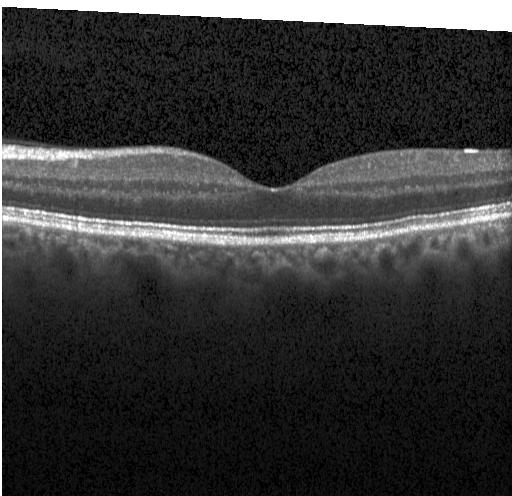 Finding: no evidence of CNV, DME, or drusen.